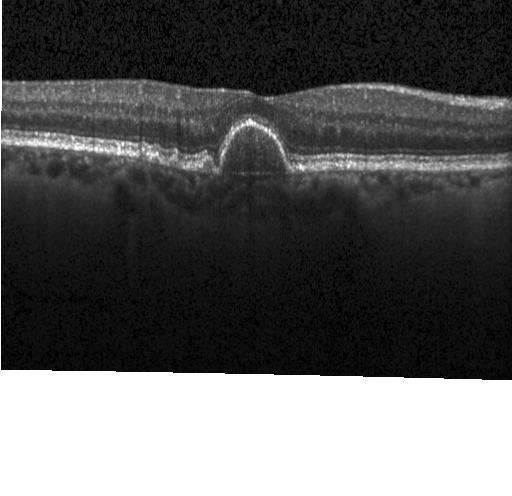
Acquired on a Heidelberg Spectralis. Centered on the fovea. Spectral-domain OCT. Retinal OCT B-scan.
Diagnosis: CNV.